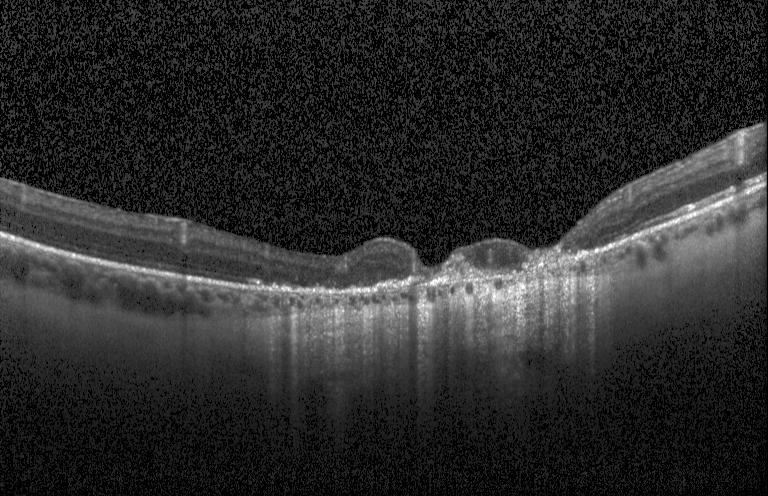

OCT B-scan
This B-scan demonstrates CNV.